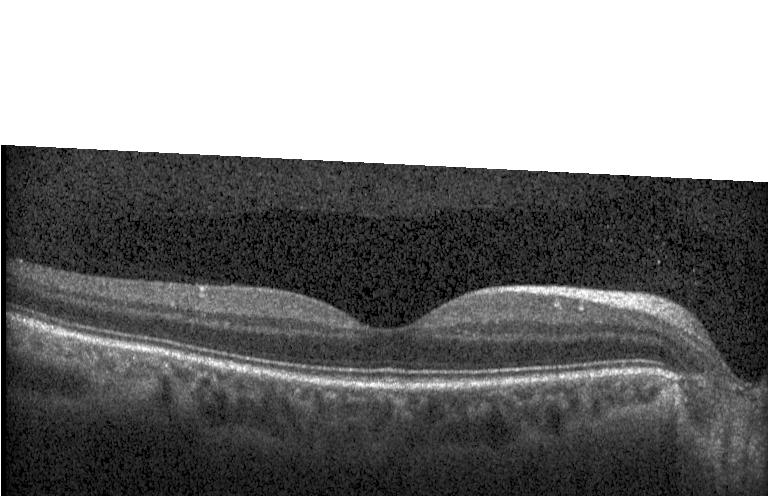

OCT B-scan showing no choroidal neovascularization, diabetic macular edema, or drusen.